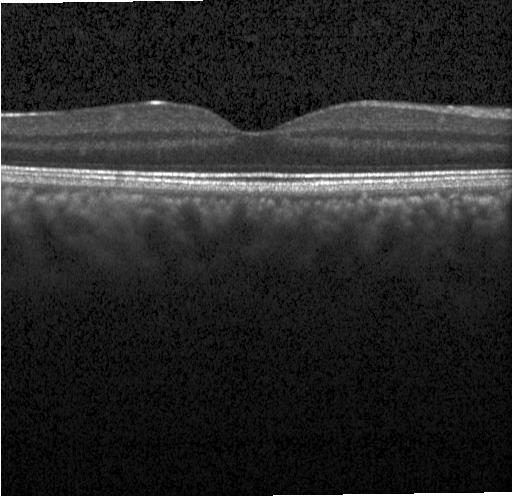

Optical coherence tomography scan, SD-OCT
Impression: no evidence of choroidal neovascularization, diabetic macular edema, or drusen.